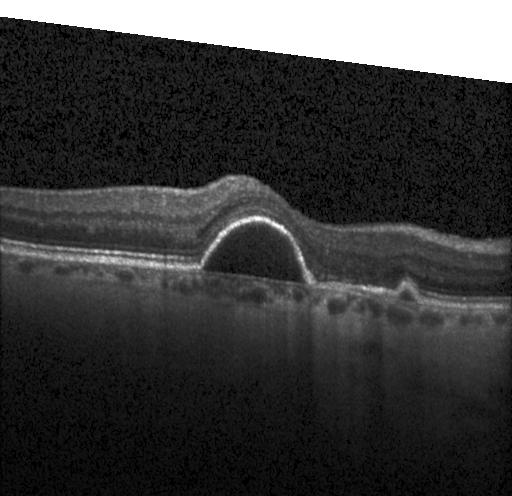 Impression: choroidal neovascularization.